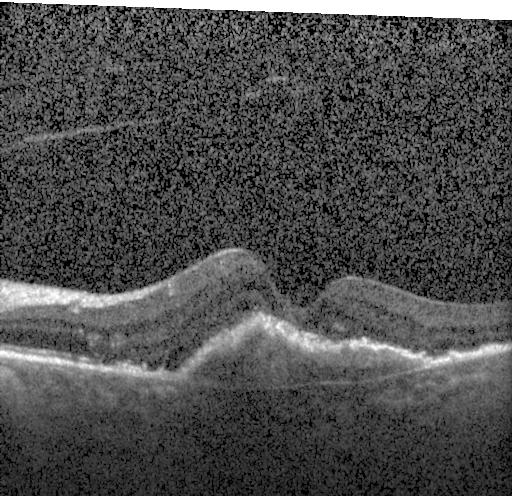

Heidelberg Spectralis, retinal OCT B-scan. This B-scan demonstrates CNV.